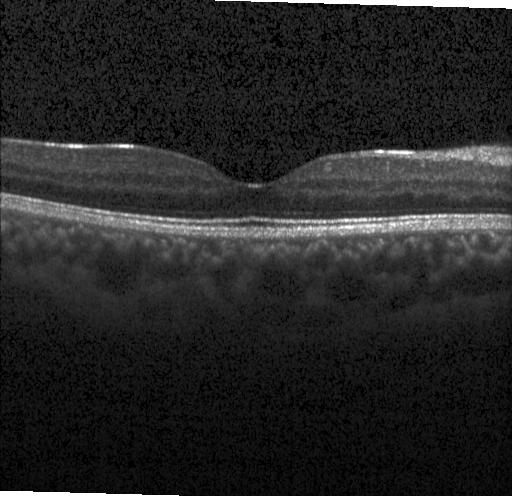

Dx: no choroidal neovascularization, diabetic macular edema, or drusen.